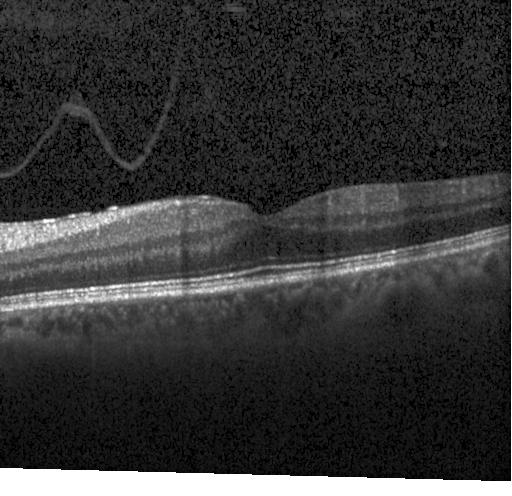 Dx: no CNV, no DME, and no drusen.